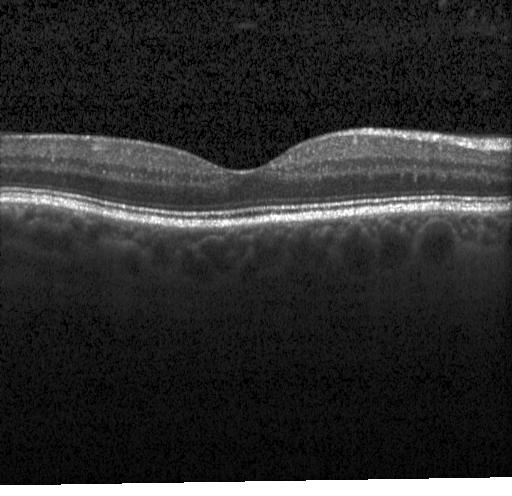 SD-OCT, Heidelberg Spectralis, macular scan, optical coherence tomography B-scan — Finding: no choroidal neovascularization, diabetic macular edema, or drusen.